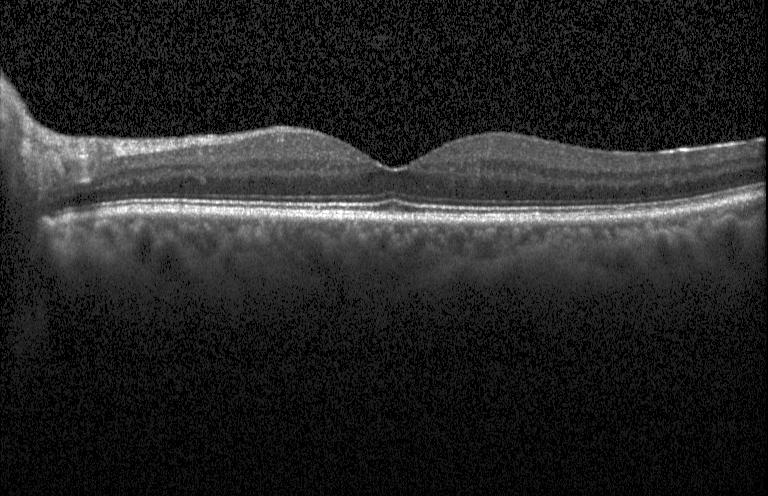
Assessment: no CNV, DME, or drusen.